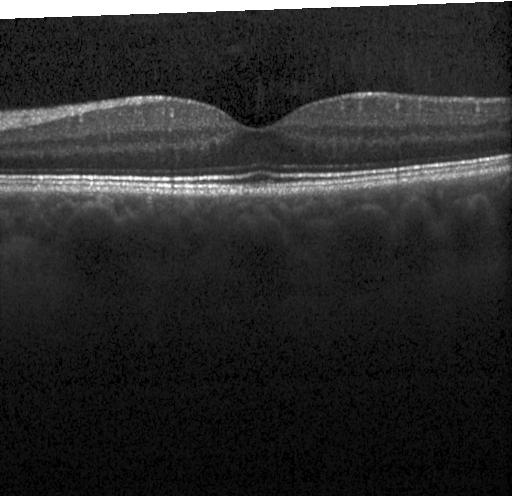
No evidence of choroidal neovascularization, diabetic macular edema, or drusen.